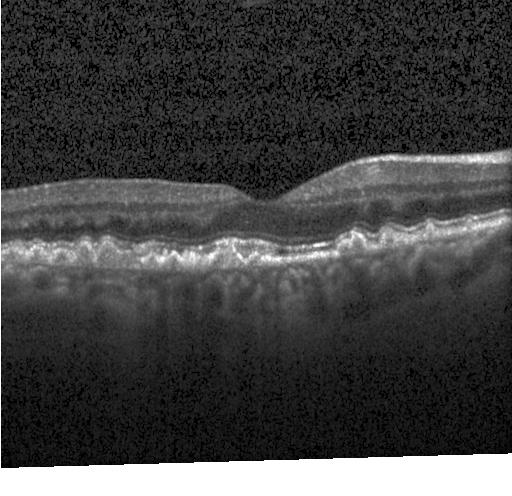
Retinal OCT B-scan
Finding: sub-RPE drusenoid deposits.